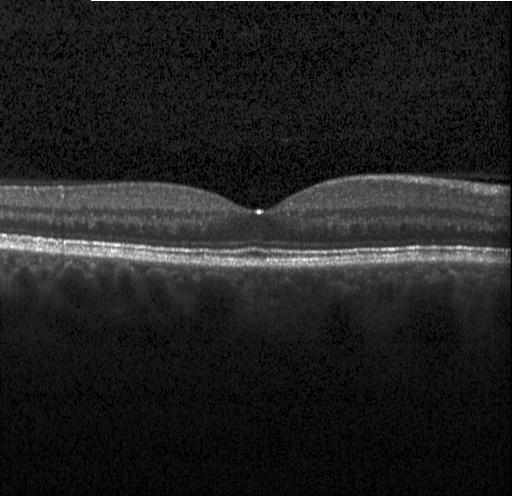
OCT B-scan — Assessment: neither choroidal neovascularization, diabetic macular edema, nor drusen.